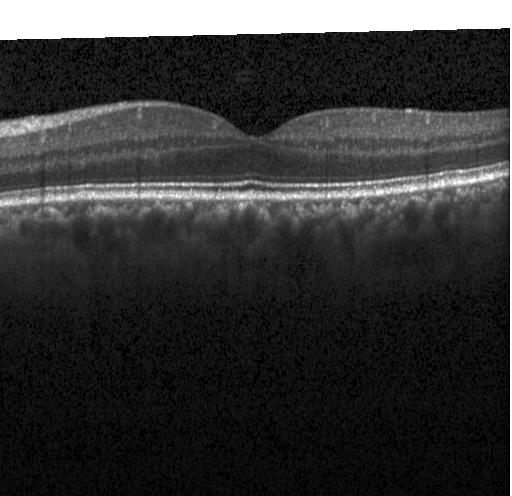
Macular OCT demonstrating no evidence of choroidal neovascularization, diabetic macular edema, or drusen.